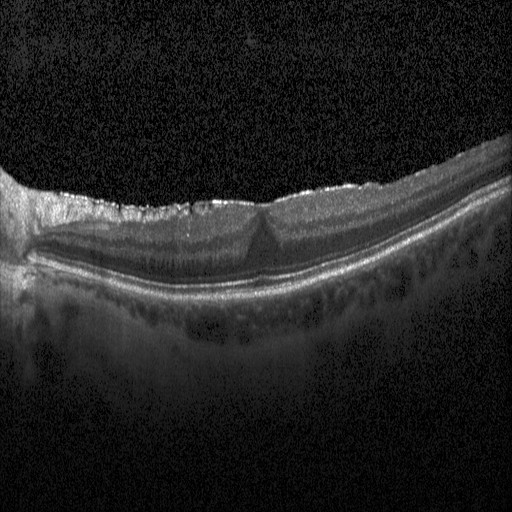
Spectral-domain optical coherence tomography · instrument: Heidelberg Spectralis · retinal OCT cross-section — Impression: diabetic macular edema.